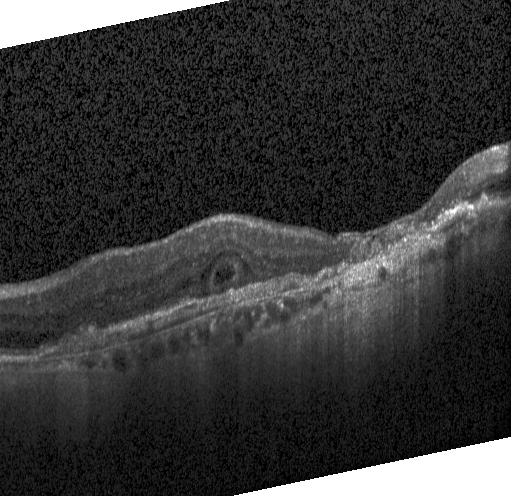

Macular OCT demonstrating choroidal neovascularization (CNV).